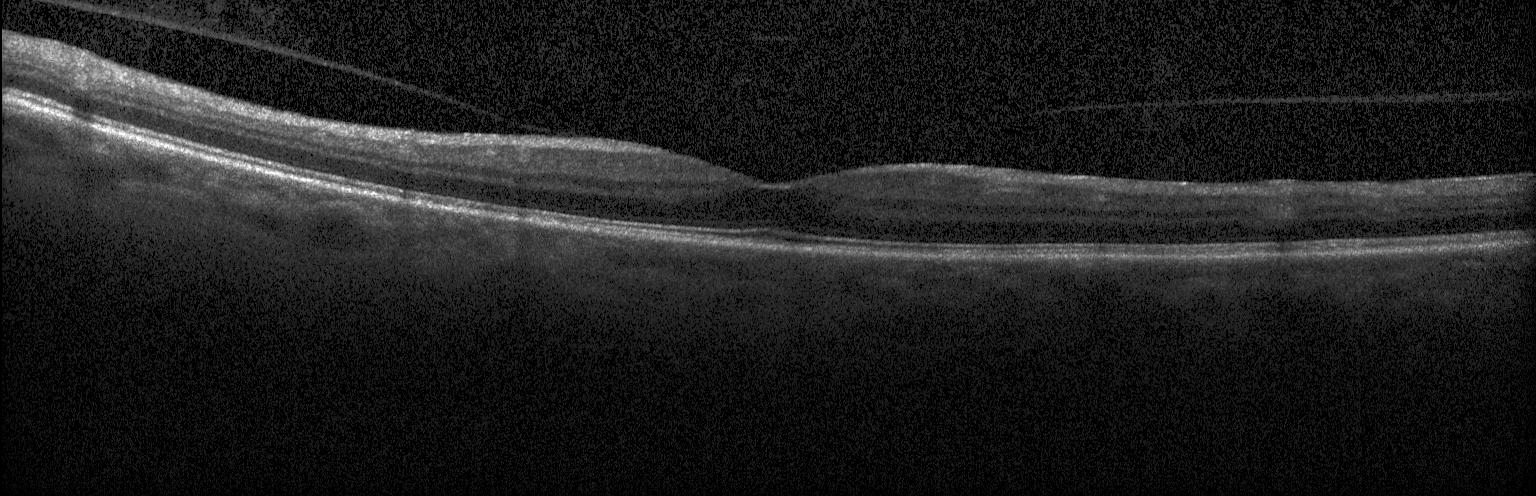 Dx: neither choroidal neovascularization, diabetic macular edema, nor drusen.